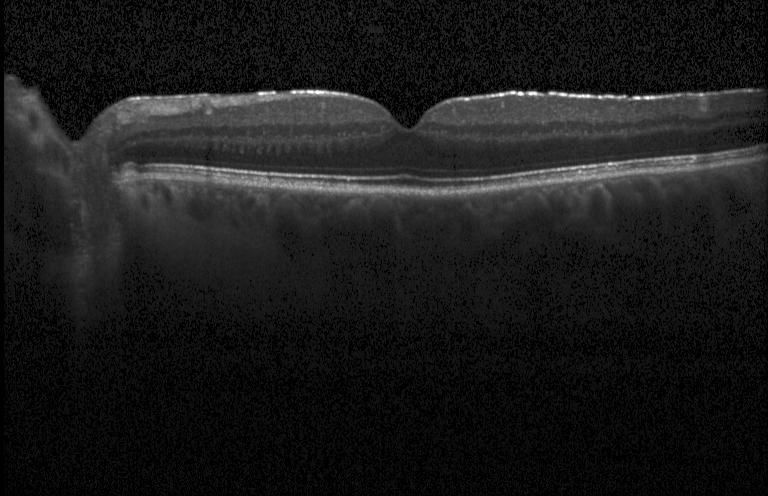
Fovea-centered, Heidelberg Spectralis, OCT line scan
Assessment: no choroidal neovascularization, no diabetic macular edema, and no drusen.